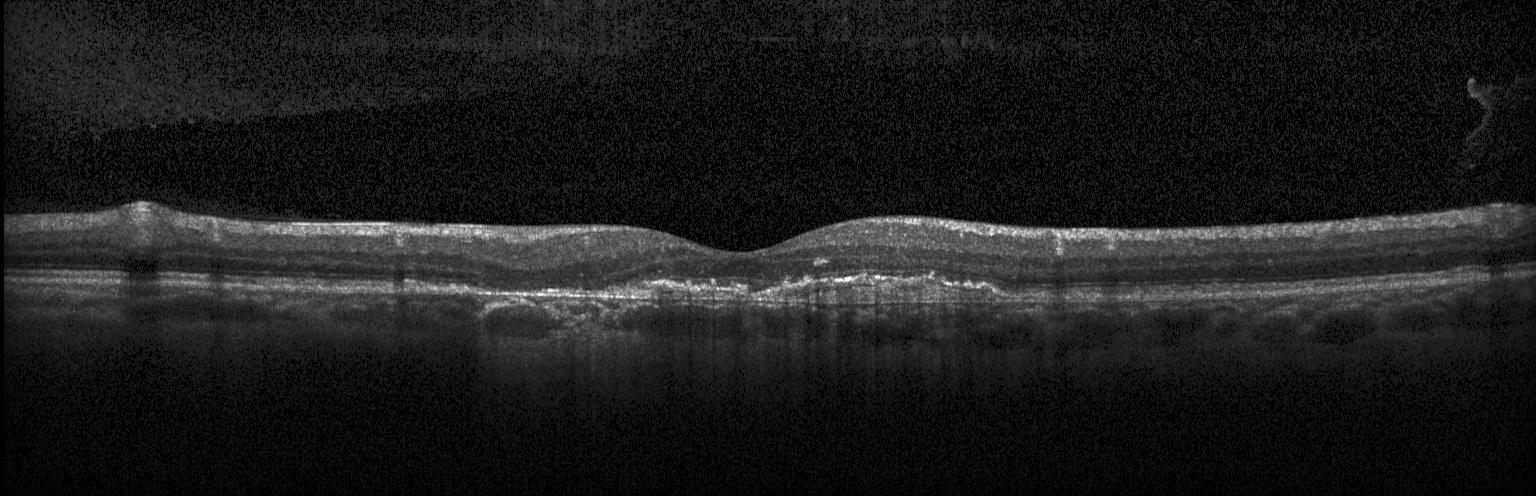 OCT B-scan.
Finding: CNV.